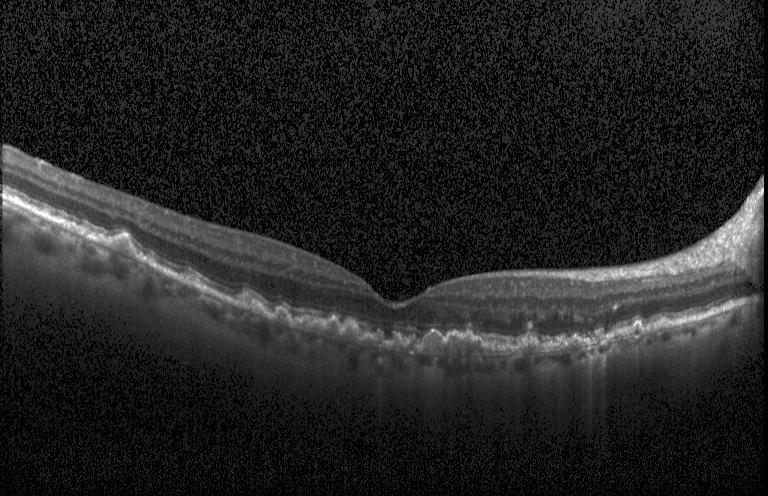

Centered on the fovea. OCT line scan. SD-OCT — This B-scan demonstrates drusen.